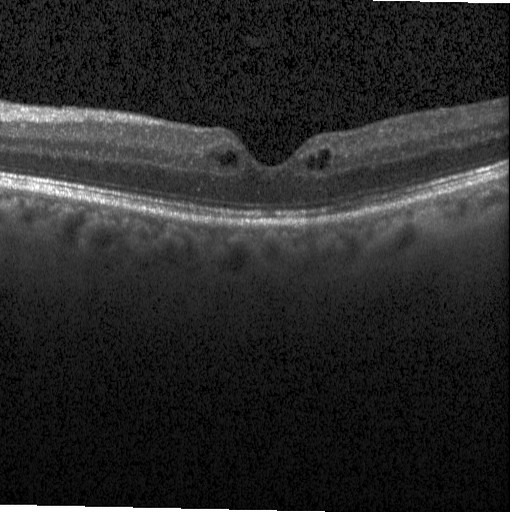 Fovea-centered, Heidelberg Spectralis OCT system, retinal OCT cross-section. Finding: DME.